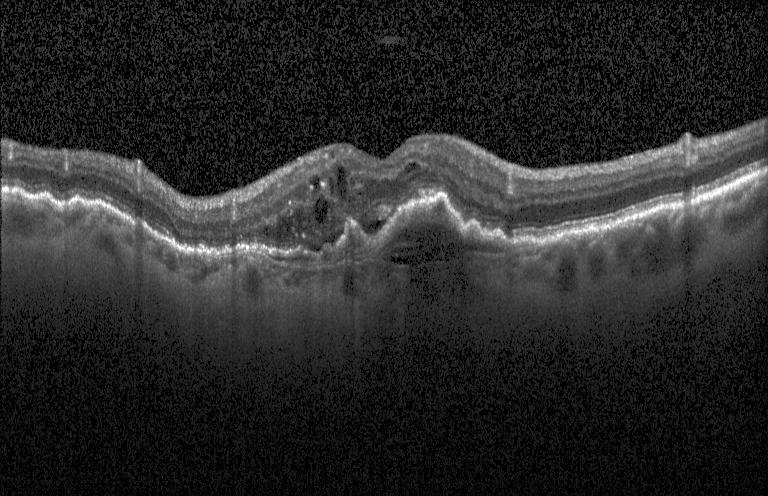

Macular OCT demonstrating choroidal neovascularization.